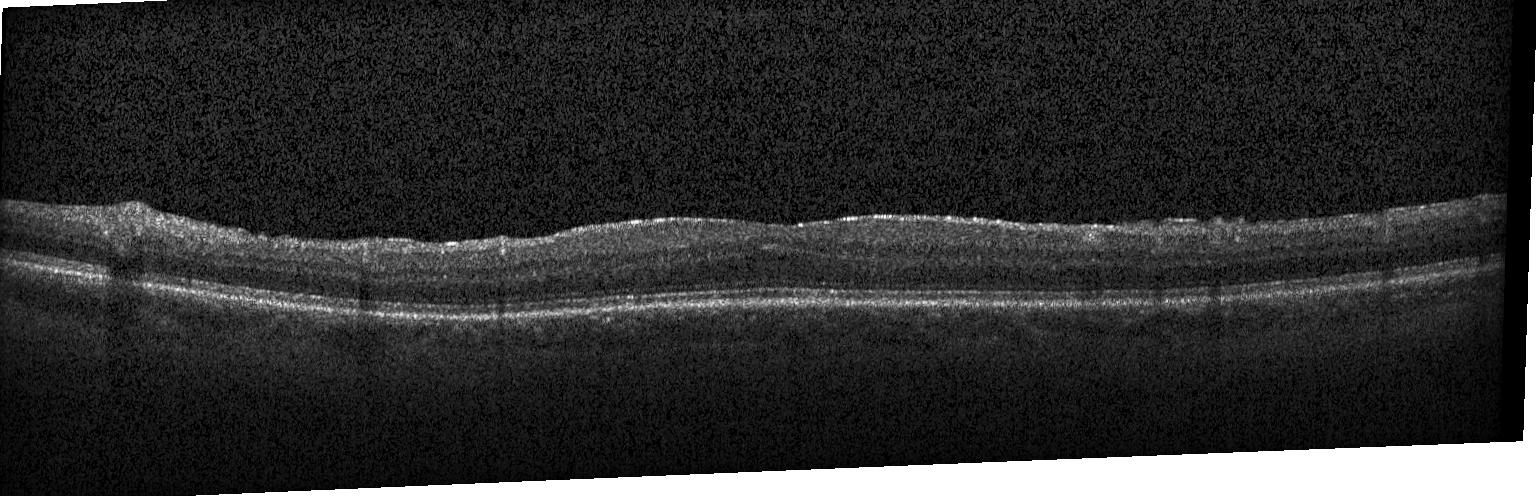

Spectral-domain OCT B-scan: no choroidal neovascularization, diabetic macular edema, or drusen.